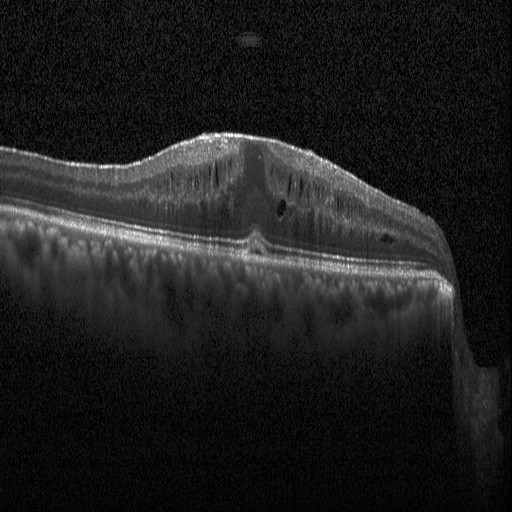

Spectral-domain optical coherence tomography, optical coherence tomography scan, Heidelberg Spectralis, macular scan.
Diagnosis: DME.